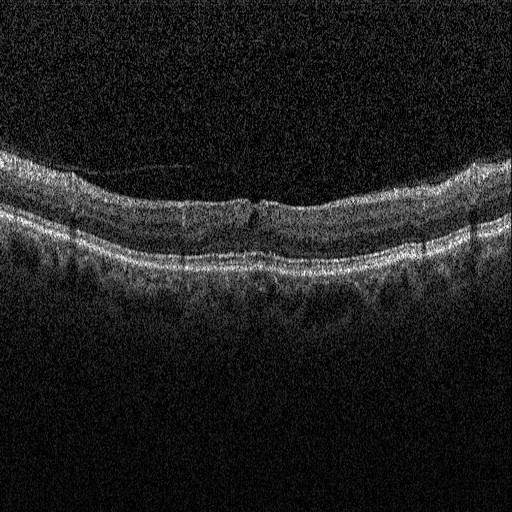
Retinal OCT cross-section showing DME.